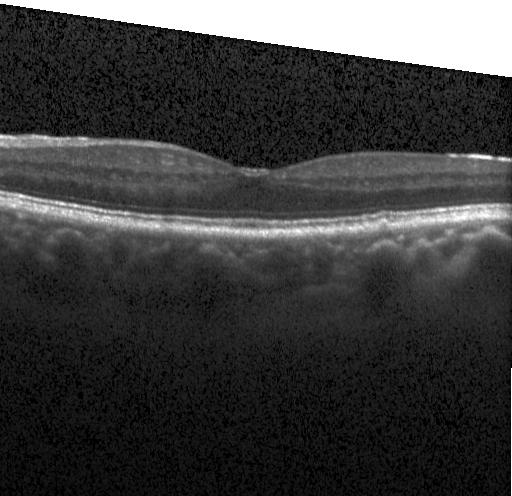
Heidelberg Spectralis OCT system · optical coherence tomography B-scan.
Finding: drusen.